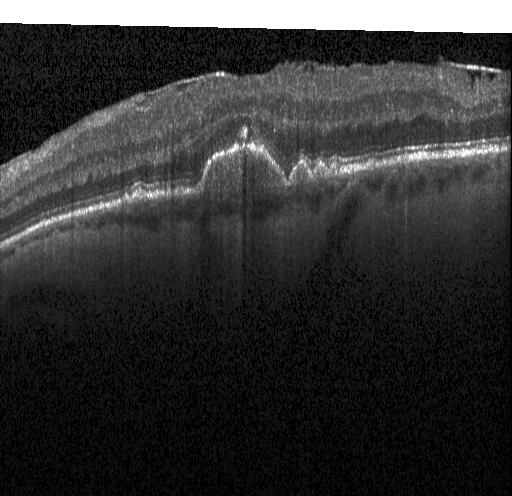

Sub-RPE drusenoid deposits.